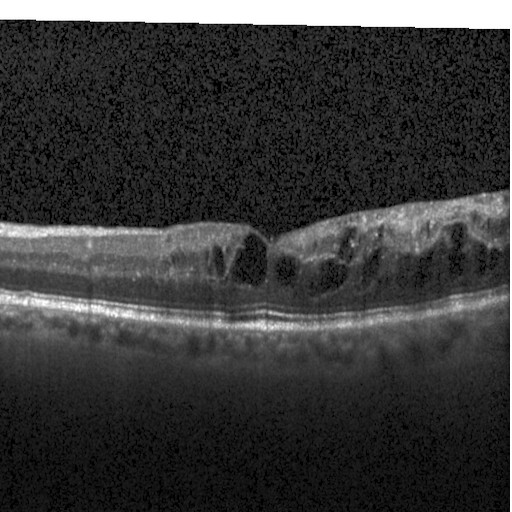
Dx: DME.